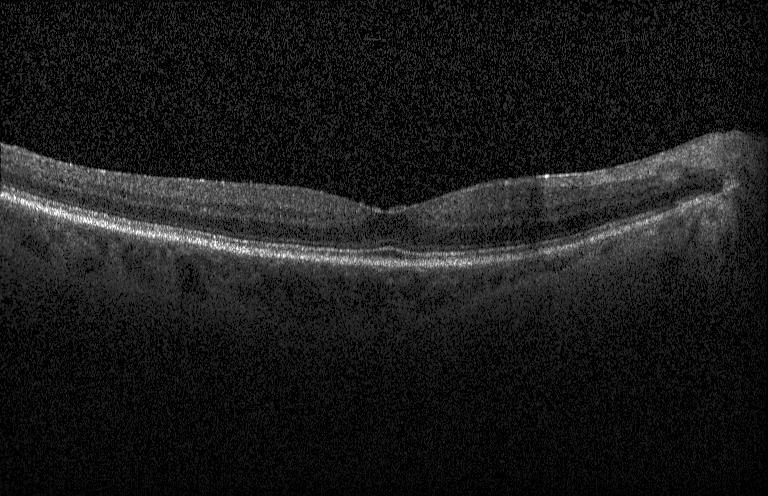

Retinal OCT B-scan
Impression: no choroidal neovascularization, diabetic macular edema, or drusen.